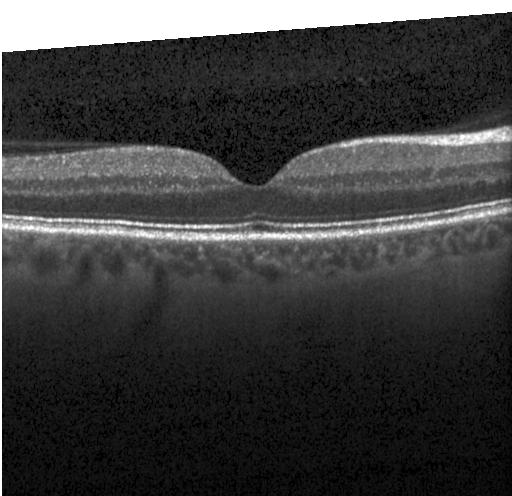
Retinal OCT cross-section. This B-scan demonstrates neither CNV, DME, nor drusen.